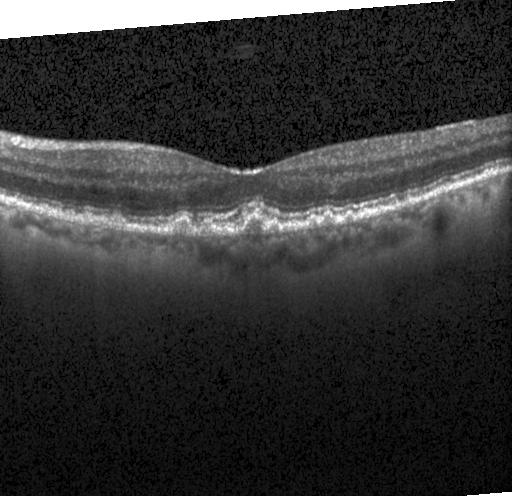
Dx: multiple drusen.